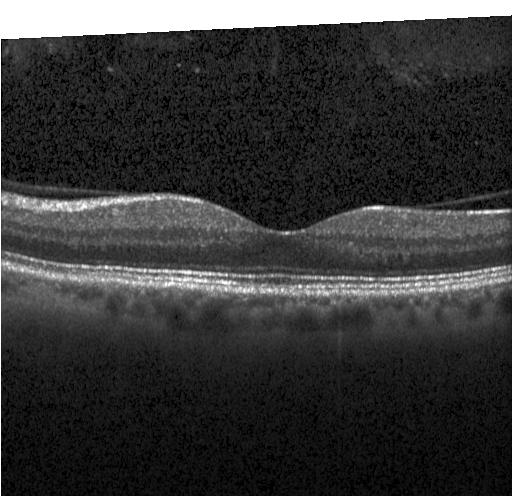
Impression: no choroidal neovascularization, diabetic macular edema, or drusen.